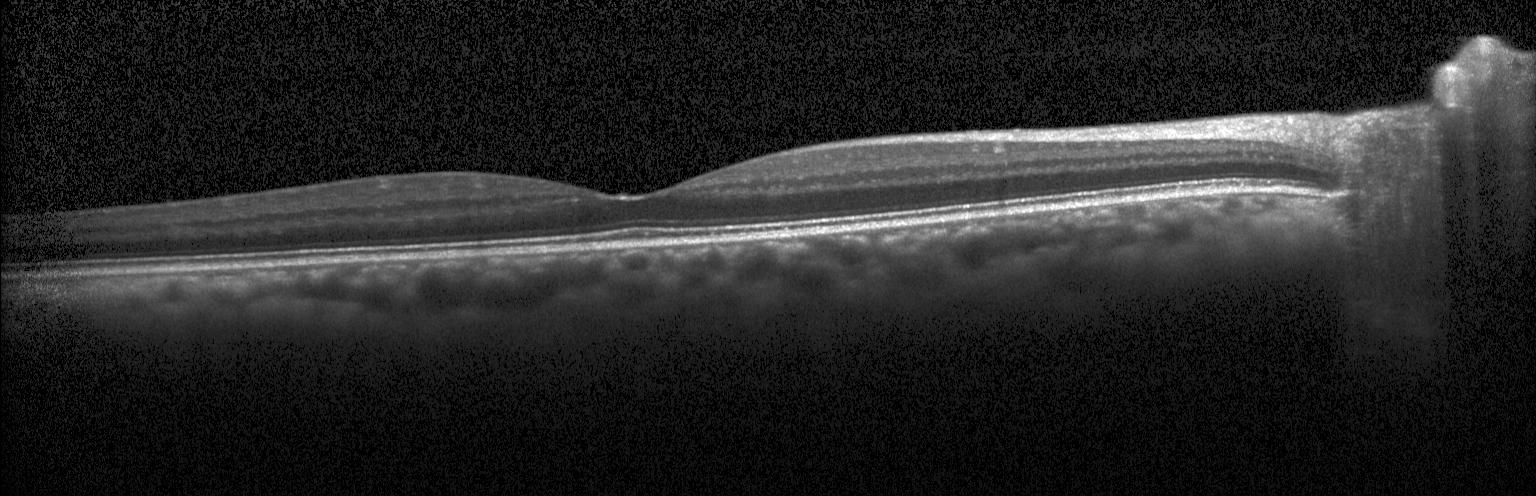 Diagnosis: no choroidal neovascularization, no diabetic macular edema, and no drusen.